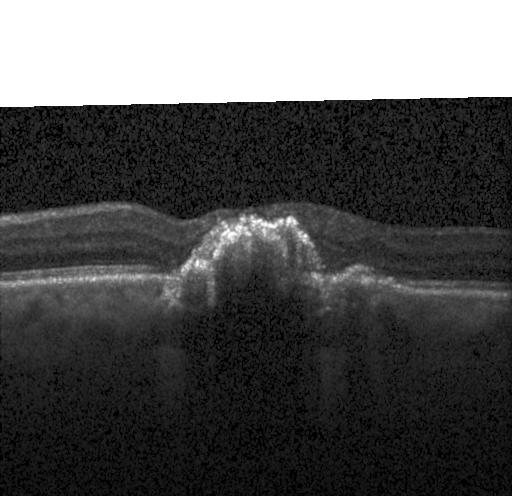

Fovea-centered; retinal OCT B-scan.
Diagnosis: a choroidal neovascular membrane.